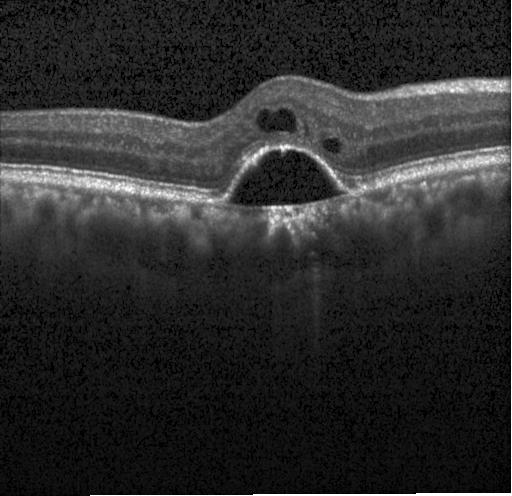

Macular OCT: a choroidal neovascular membrane.